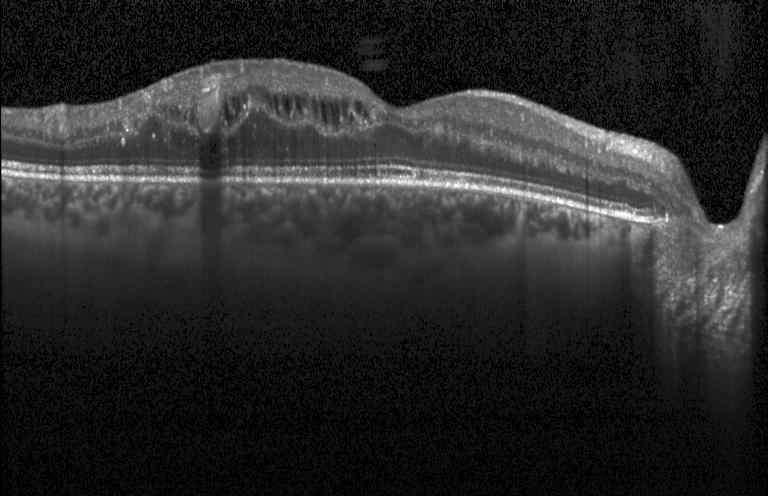

OCT finding: DME.